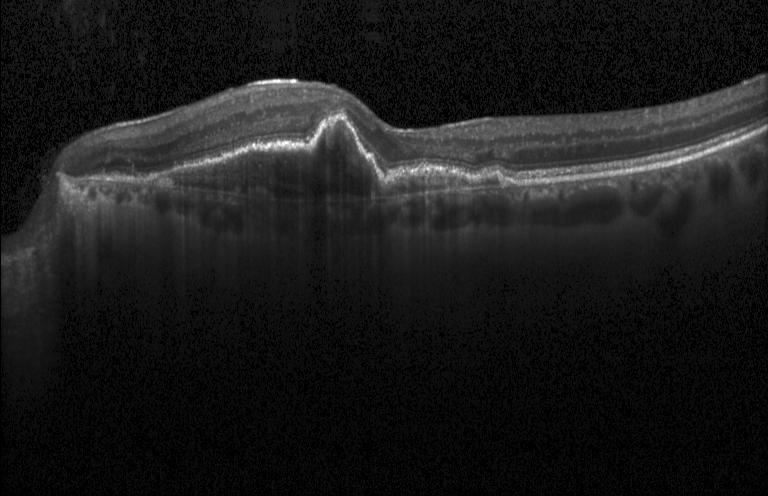
Retinal OCT B-scan · spectral-domain OCT — Finding: a choroidal neovascular membrane.